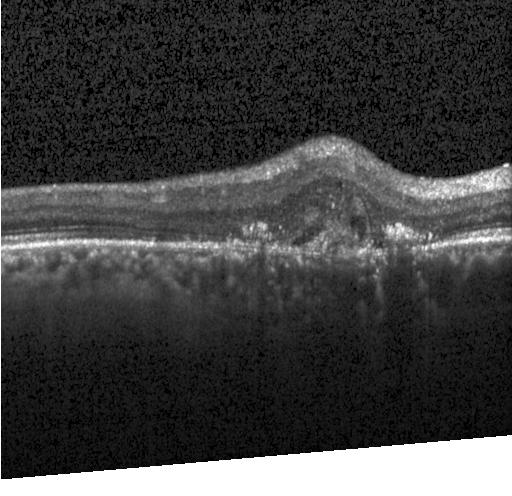
Retinal OCT B-scan. Heidelberg Spectralis OCT system. The scan shows choroidal neovascularization (CNV).